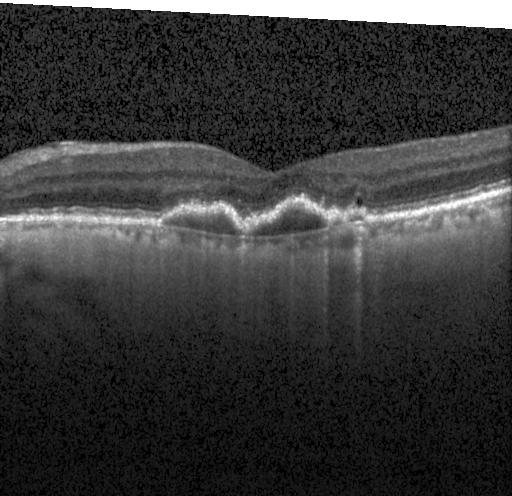
Macular scan, retinal OCT B-scan, SD-OCT — OCT finding: choroidal neovascularization (CNV).